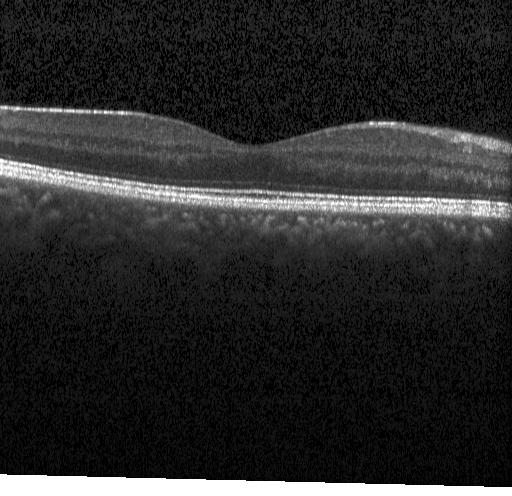 Diagnosis: no CNV, DME, or drusen.